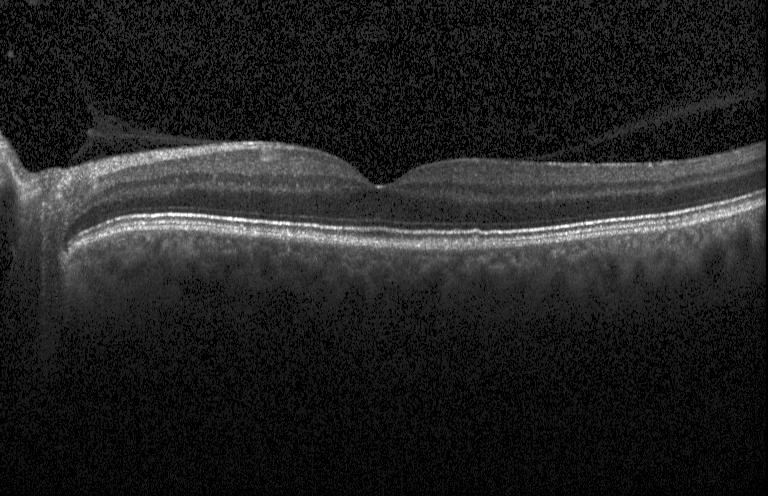

Assessment: no evidence of choroidal neovascularization, diabetic macular edema, or drusen.